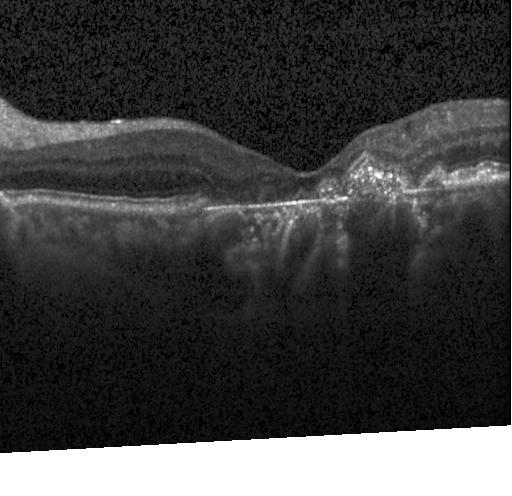
Through the macula; retinal OCT B-scan — Impression: CNV.